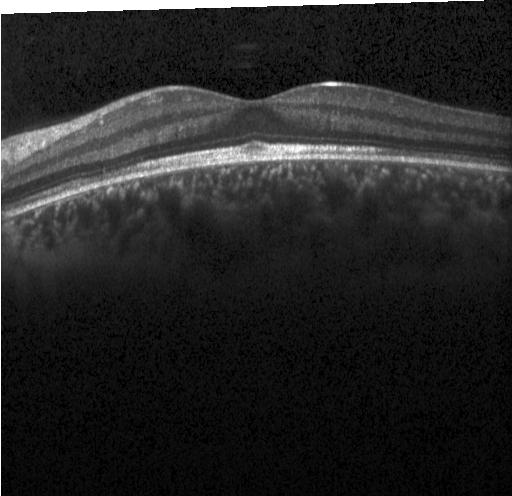

Through the macula · retinal OCT cross-section · spectral-domain OCT · instrument: Heidelberg Spectralis. Impression: no evidence of choroidal neovascularization, diabetic macular edema, or drusen.